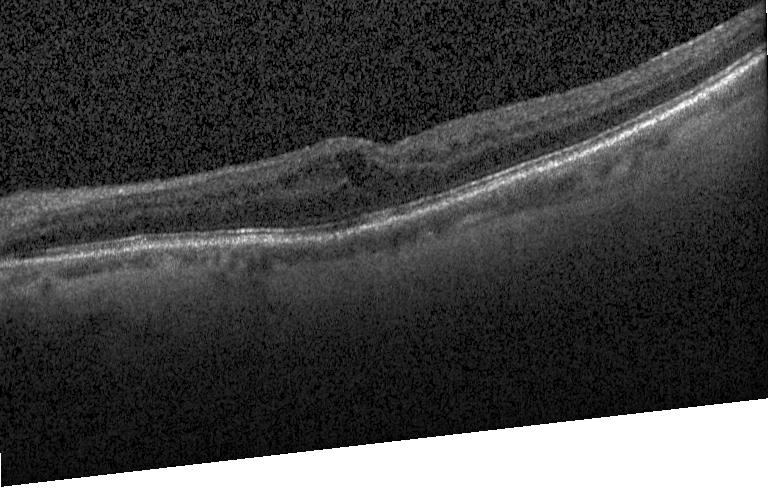 This B-scan demonstrates diabetic macular edema (DME).